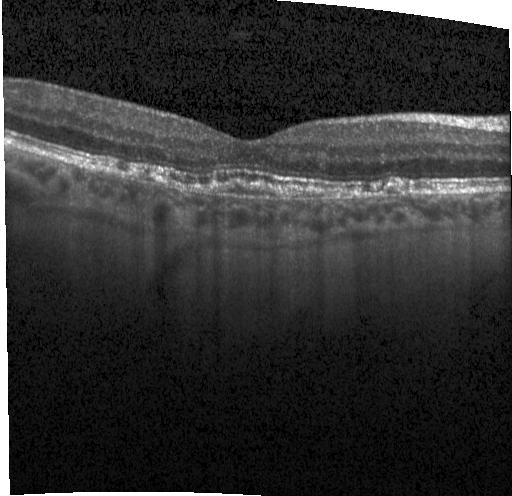
Heidelberg Spectralis. Optical coherence tomography B-scan. Diagnosis: a choroidal neovascular membrane.